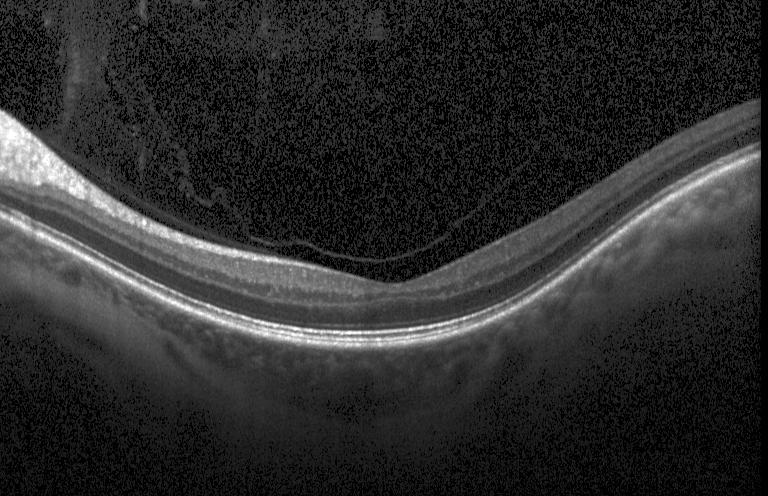 Finding: no evidence of CNV, DME, or drusen.